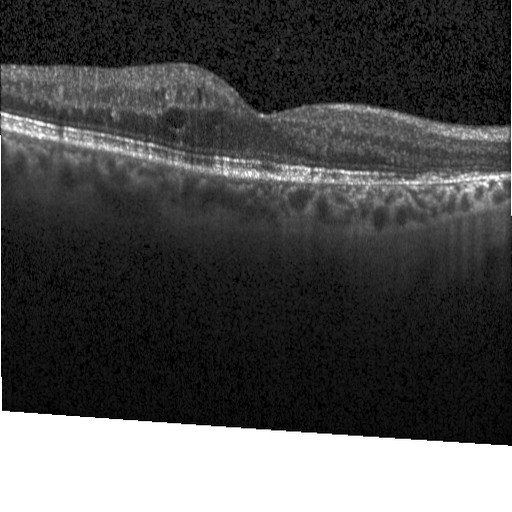

OCT B-scan — Dx: DME.